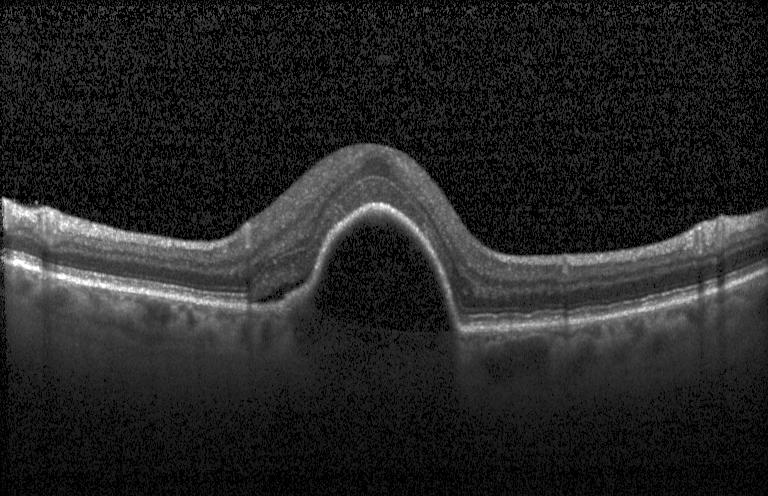

Optical coherence tomography scan.
Impression: a choroidal neovascular membrane.